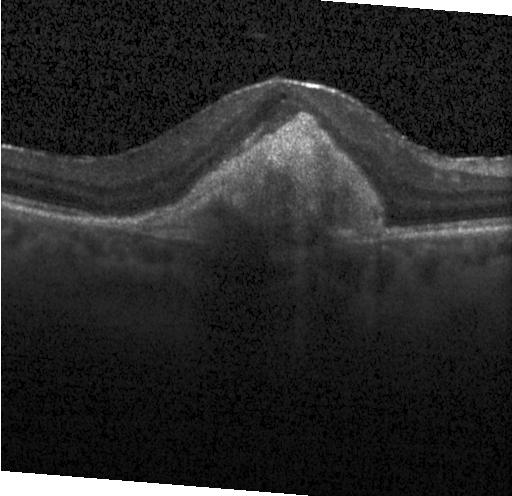 OCT scan showing choroidal neovascularization.